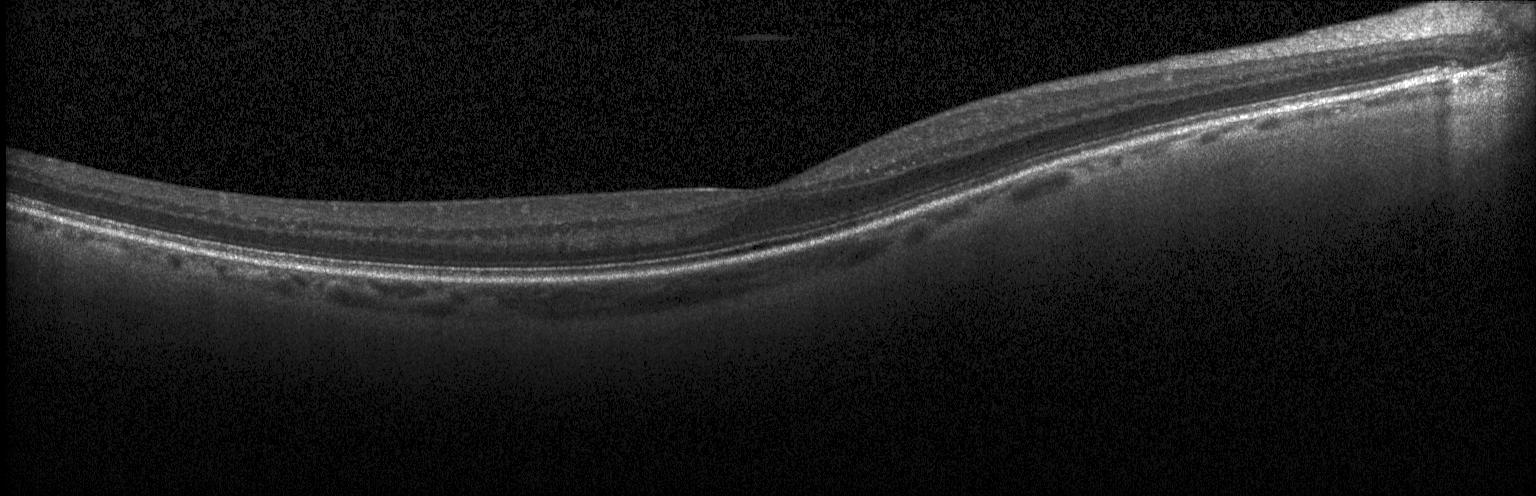

Through the macula · spectral-domain optical coherence tomography · Heidelberg Spectralis · optical coherence tomography B-scan — Assessment: no evidence of choroidal neovascularization, diabetic macular edema, or drusen.